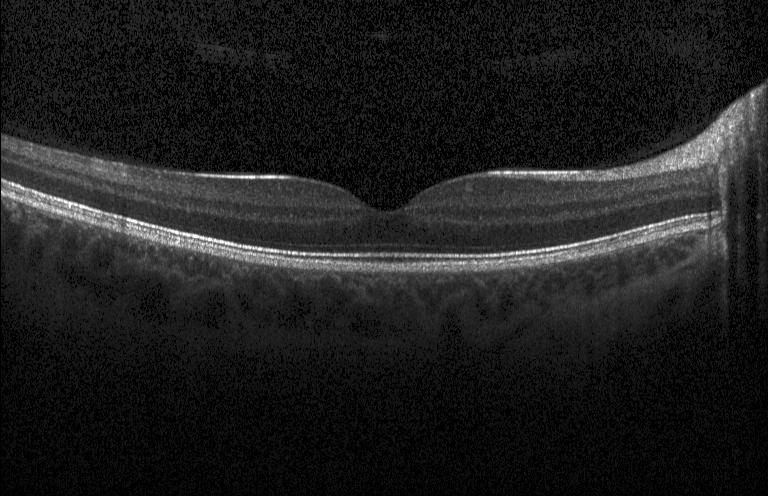

Spectral-domain OCT; instrument: Heidelberg Spectralis; retinal OCT B-scan. This B-scan demonstrates no CNV, no DME, and no drusen.